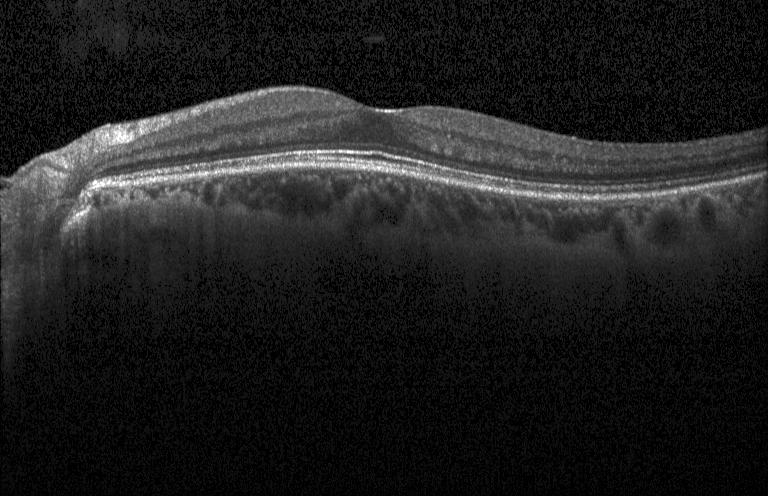
This B-scan demonstrates no evidence of CNV, DME, or drusen.